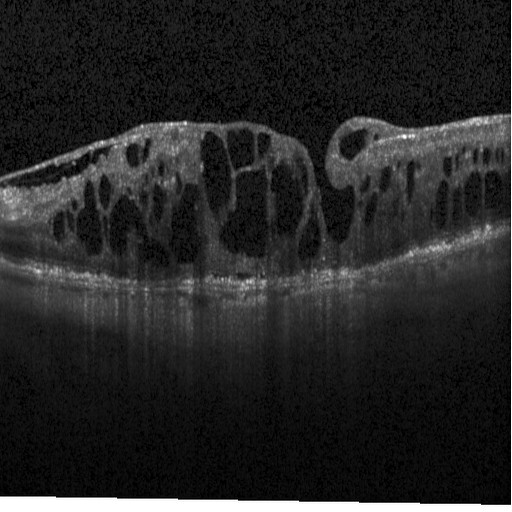

Retinal OCT cross-section showing diabetic macular edema (DME).